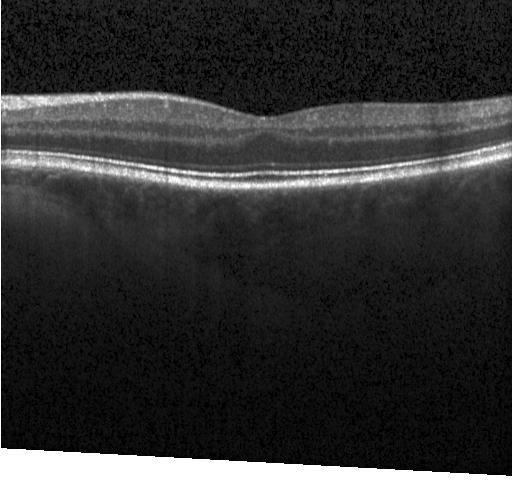

Optical coherence tomography B-scan.
Assessment: no CNV, DME, or drusen.